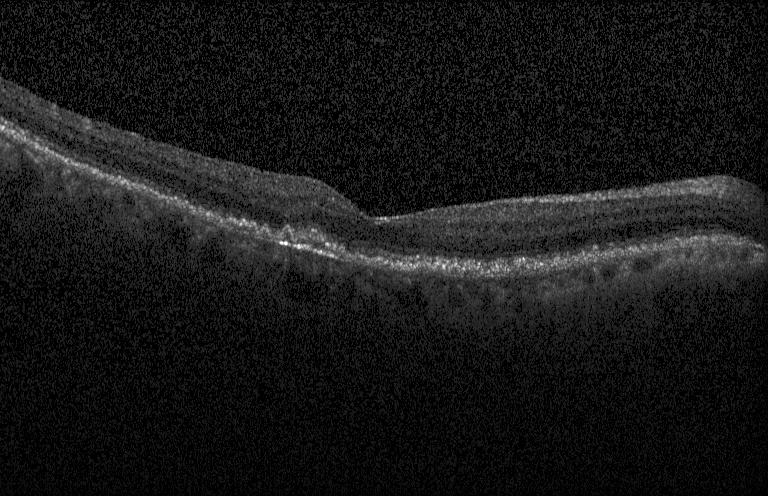
Heidelberg Spectralis OCT system; retinal OCT cross-section.
Drusen.